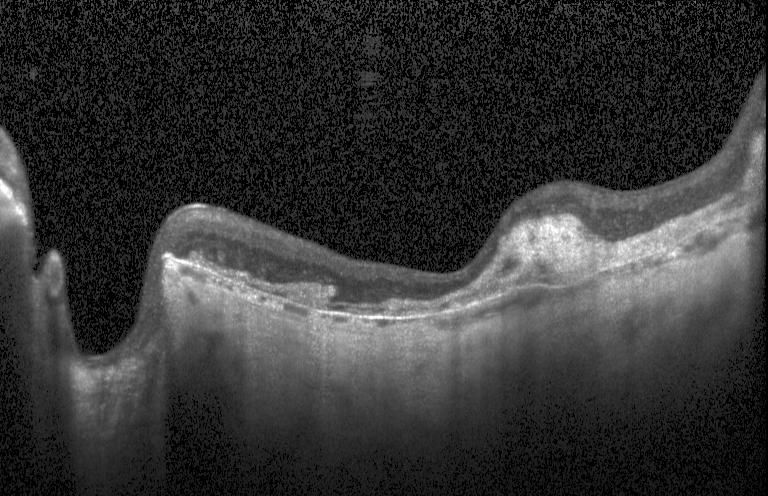 Assessment: choroidal neovascularization (CNV).